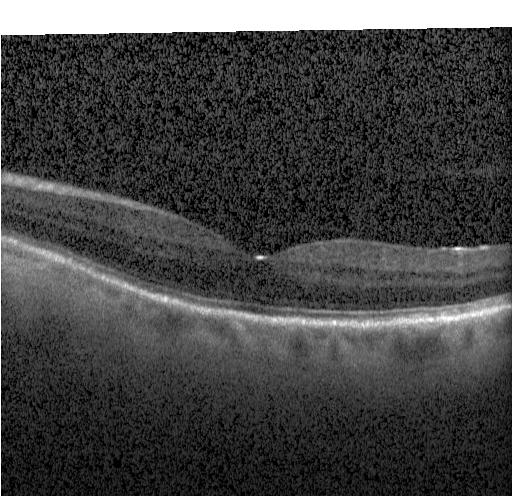

Retinal OCT cross-section showing no evidence of CNV, DME, or drusen.